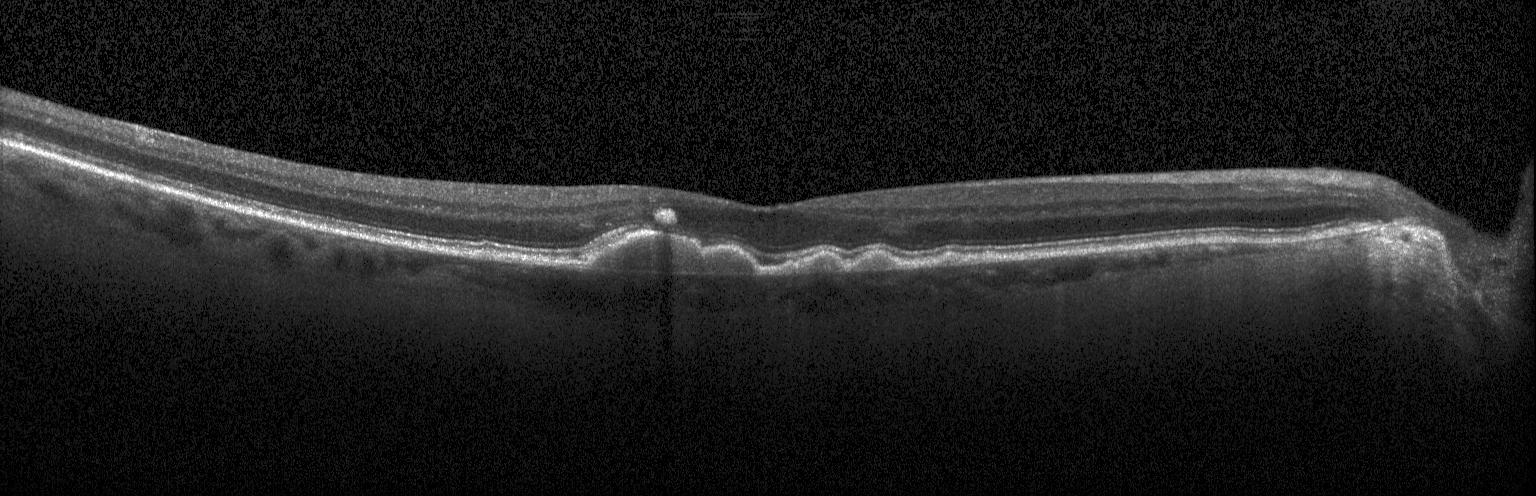 Dx: a choroidal neovascular membrane.